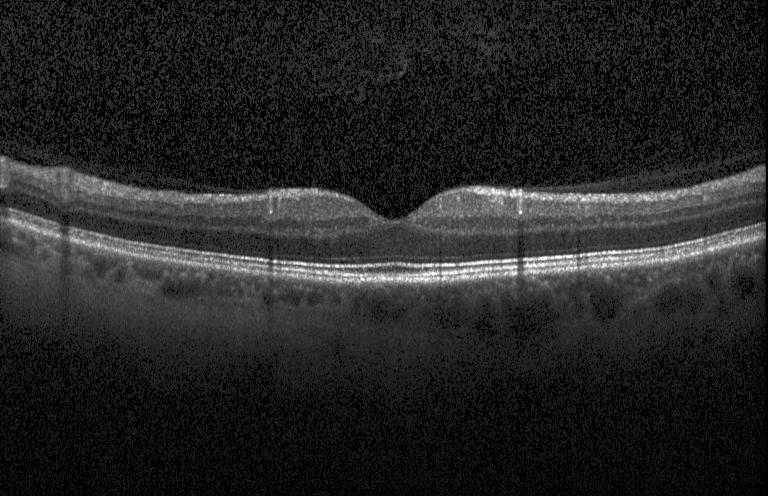

Optical coherence tomography scan. The scan shows neither choroidal neovascularization, diabetic macular edema, nor drusen.